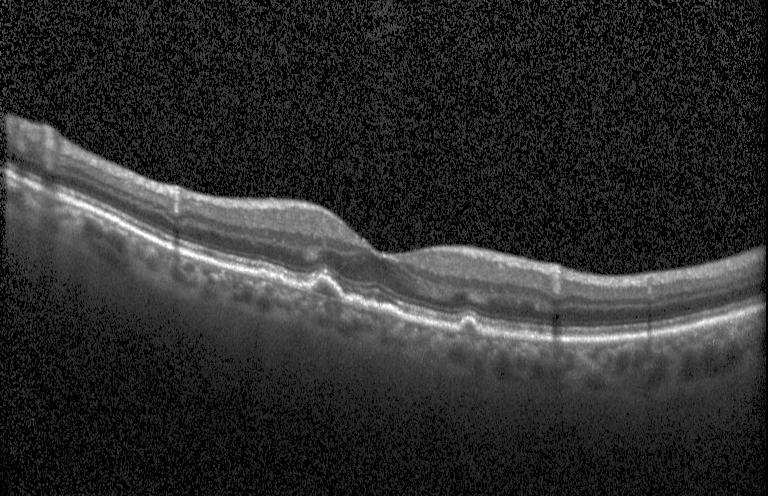
OCT B-scan showing sub-RPE drusenoid deposits.